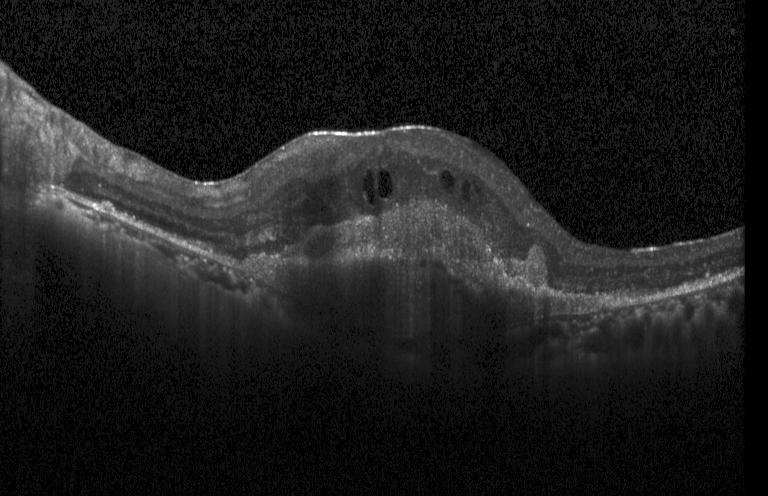
Spectral-domain optical coherence tomography; OCT line scan.
Dx: choroidal neovascularization.